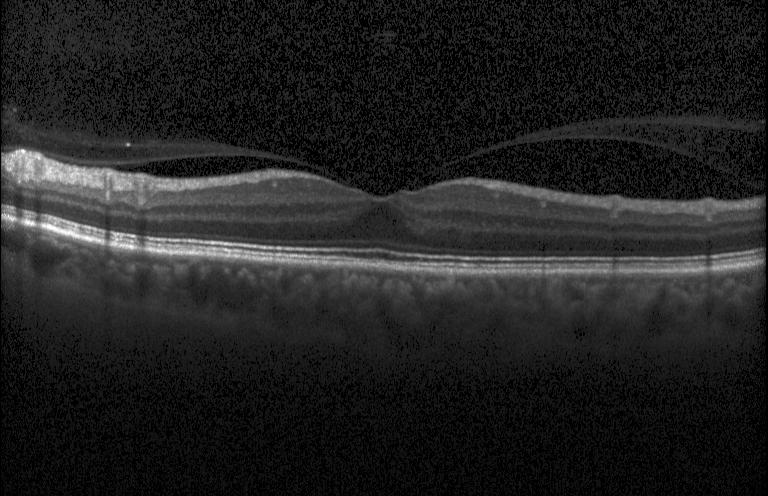
Optical coherence tomography B-scan; Heidelberg Spectralis; centered on the fovea; SD-OCT
This B-scan demonstrates neither choroidal neovascularization, diabetic macular edema, nor drusen.